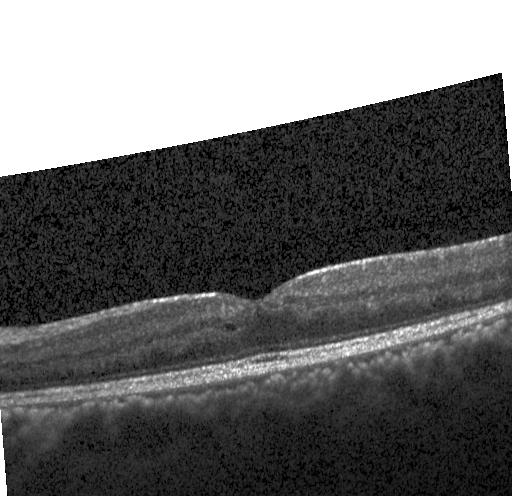

Spectral-domain OCT, centered on the fovea, OCT line scan, Heidelberg Spectralis OCT system.
Dx: diabetic macular edema.